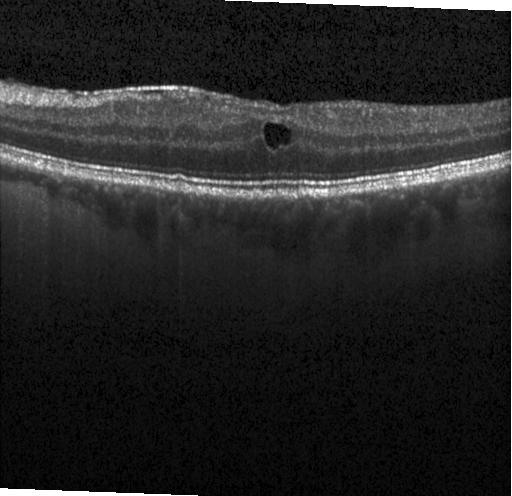

Centered on the fovea; OCT line scan — Finding: DME.